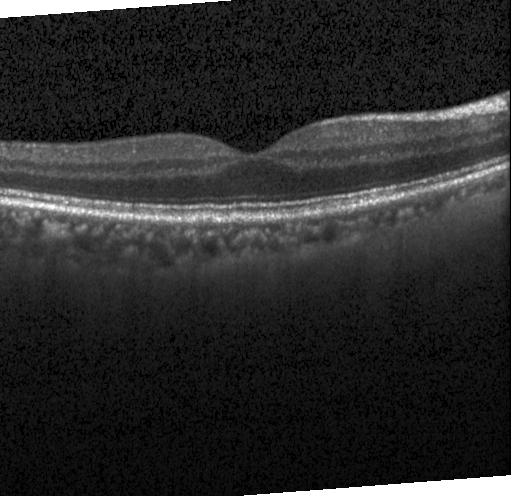
SD-OCT; OCT B-scan. No evidence of choroidal neovascularization, diabetic macular edema, or drusen.